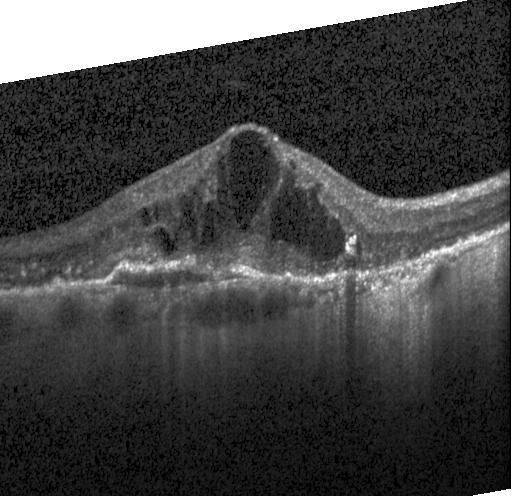
Retinal OCT B-scan · instrument: Heidelberg Spectralis · spectral-domain optical coherence tomography.
Assessment: a choroidal neovascular membrane.